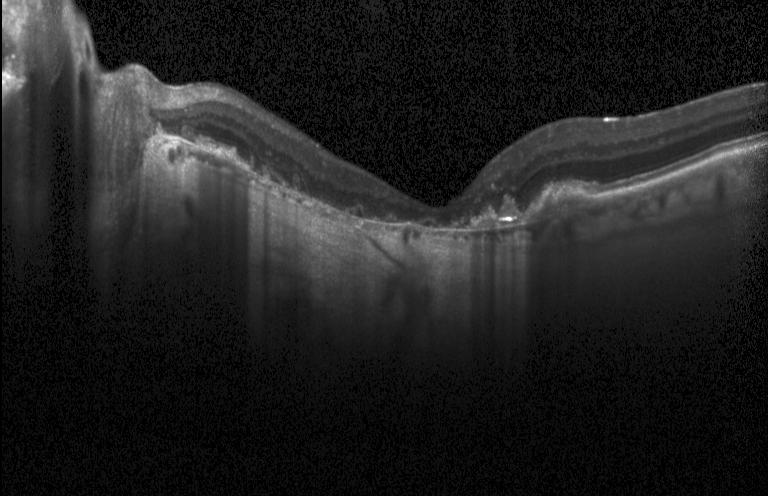
SD-OCT; horizontal scan through the fovea; Heidelberg Spectralis OCT system; OCT line scan — Diagnosis: a choroidal neovascular membrane.